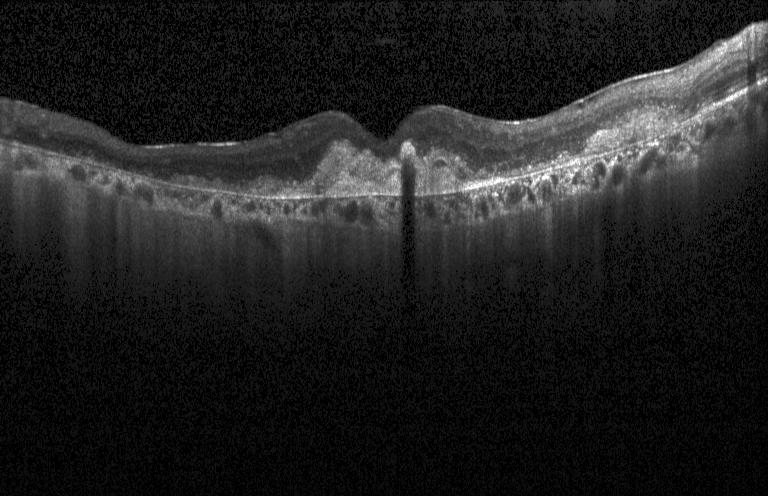
Spectral-domain OCT; Heidelberg Spectralis OCT system; retinal OCT cross-section. This B-scan demonstrates choroidal neovascularization (CNV).